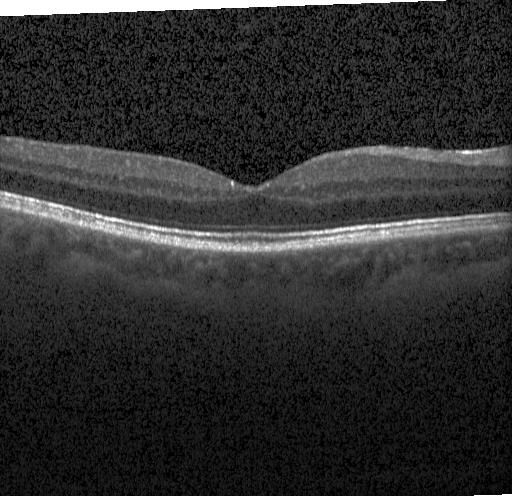

Spectral-domain OCT. Macular scan. Optical coherence tomography scan. Heidelberg Spectralis
Diagnosis: no evidence of CNV, DME, or drusen.